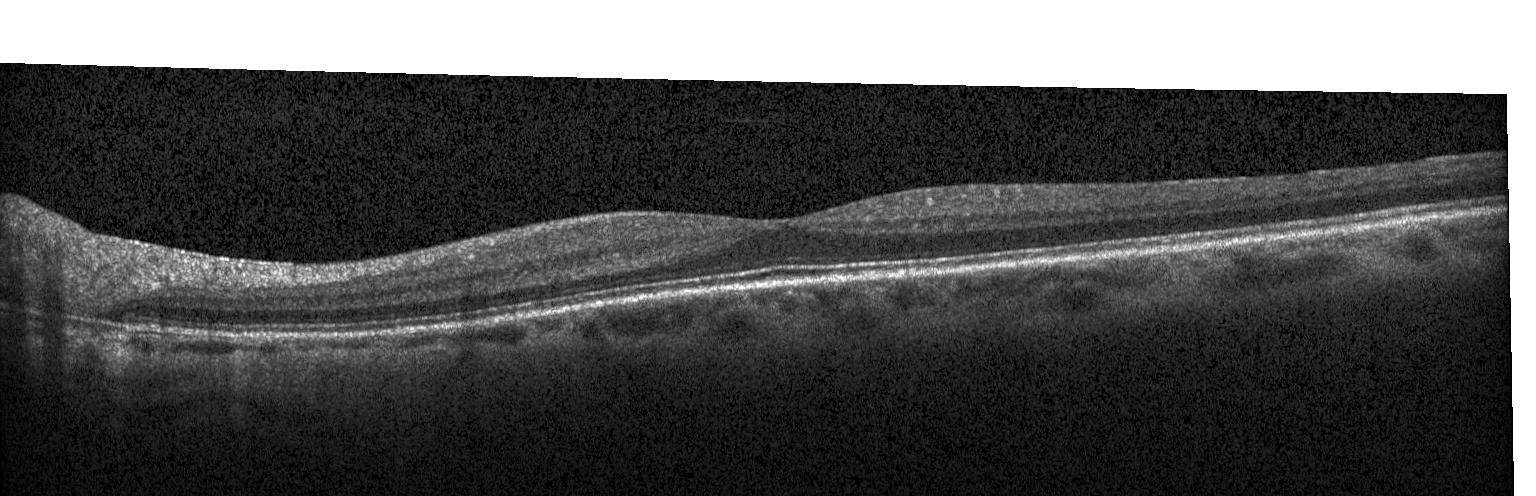 Spectral-domain optical coherence tomography, horizontal scan through the fovea, OCT line scan.
Finding: no choroidal neovascularization, diabetic macular edema, or drusen.